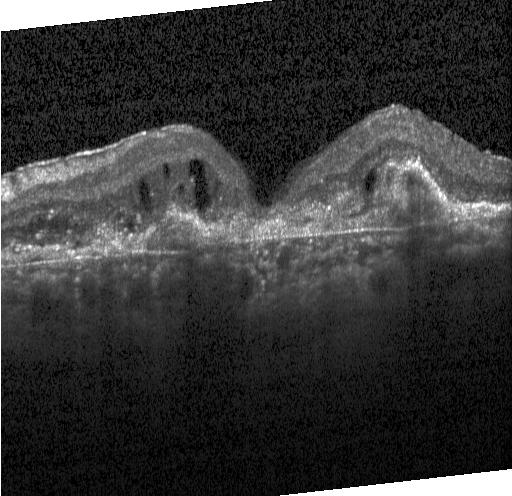
Optical coherence tomography B-scan · spectral-domain optical coherence tomography
Impression: a choroidal neovascular membrane.